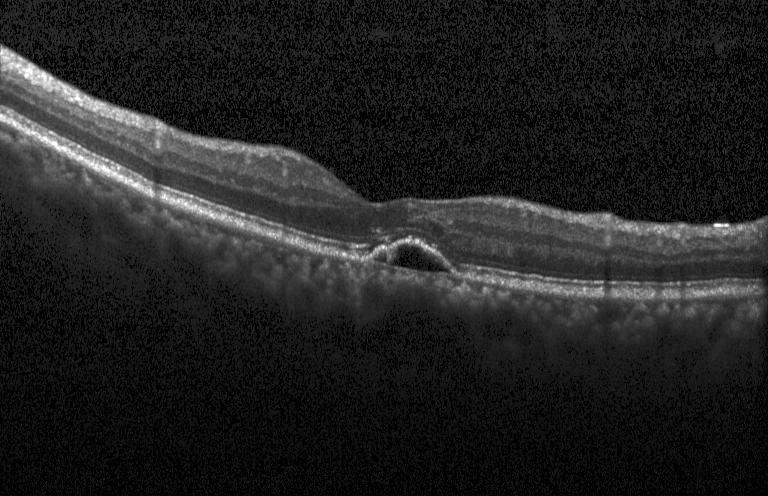

Heidelberg Spectralis OCT system; macular scan; OCT line scan. Assessment: choroidal neovascularization.